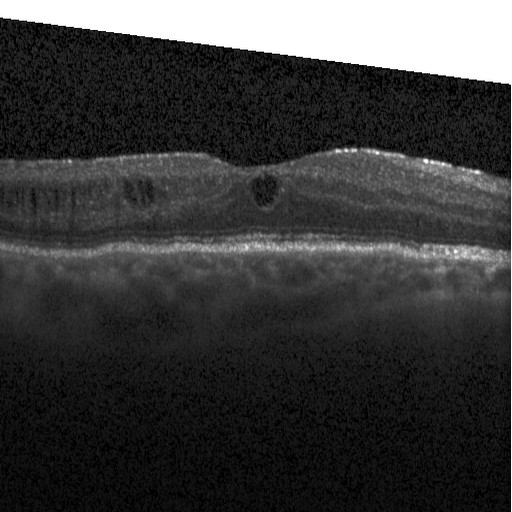

Impression: diabetic macular edema.